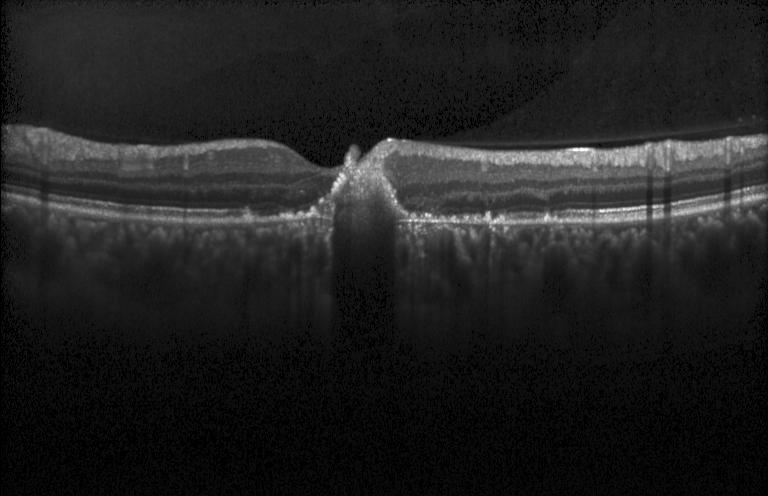 Heidelberg Spectralis OCT system. Optical coherence tomography B-scan.
Diagnosis: choroidal neovascularization.